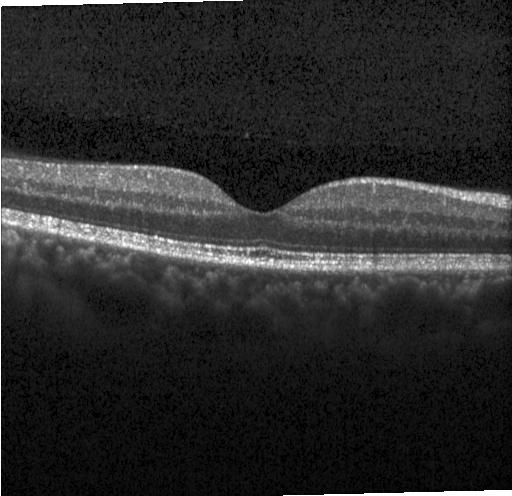
Centered on the fovea · OCT B-scan · instrument: Heidelberg Spectralis · SD-OCT
This B-scan demonstrates no CNV, DME, or drusen.